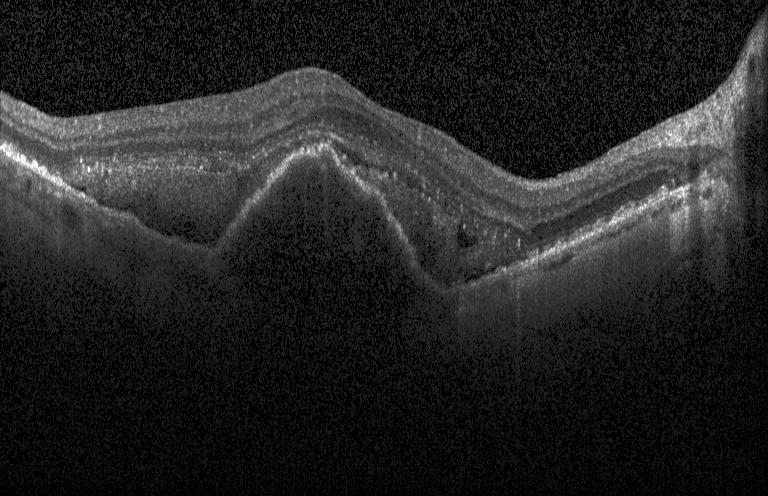

OCT line scan — CNV.